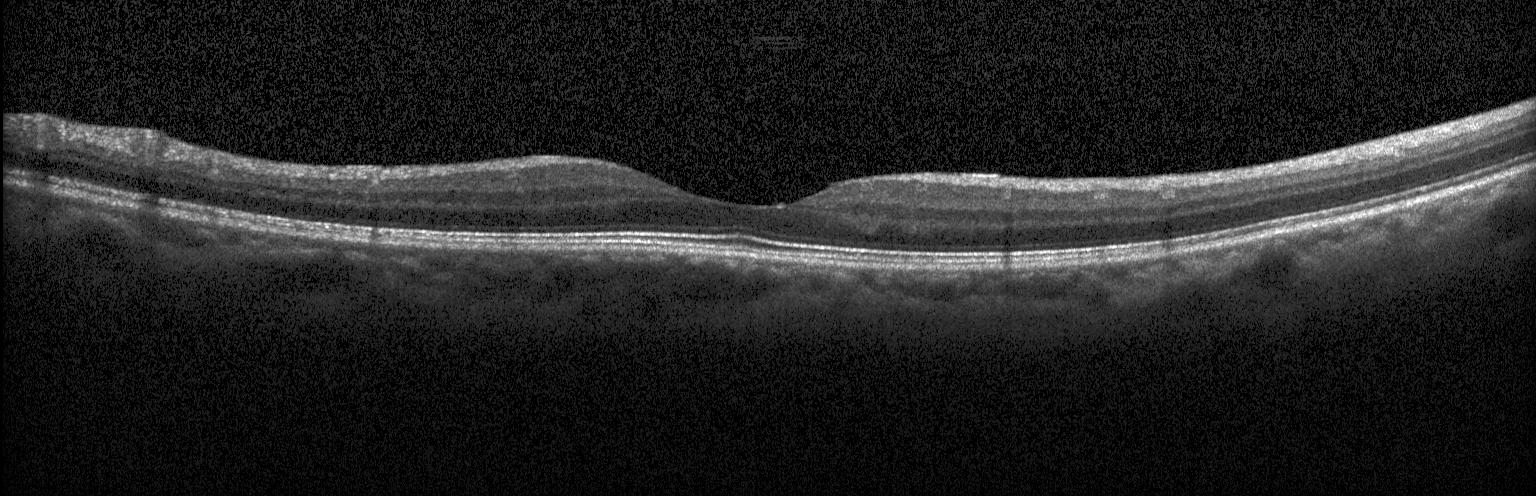 Instrument: Heidelberg Spectralis. Spectral-domain OCT. Optical coherence tomography B-scan. OCT finding: no evidence of choroidal neovascularization, diabetic macular edema, or drusen.